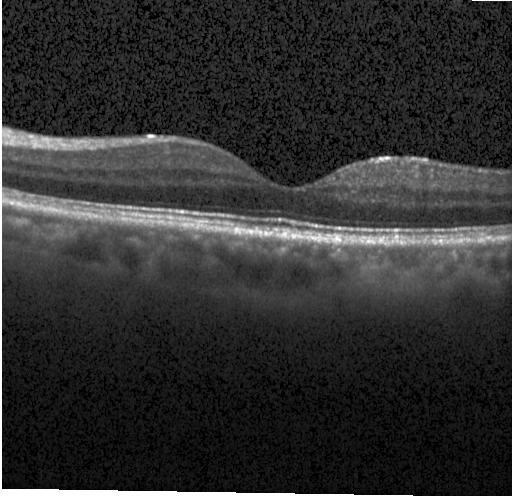
Spectral-domain optical coherence tomography. Retinal OCT B-scan. Through the macula.
Diagnosis: no evidence of CNV, DME, or drusen.